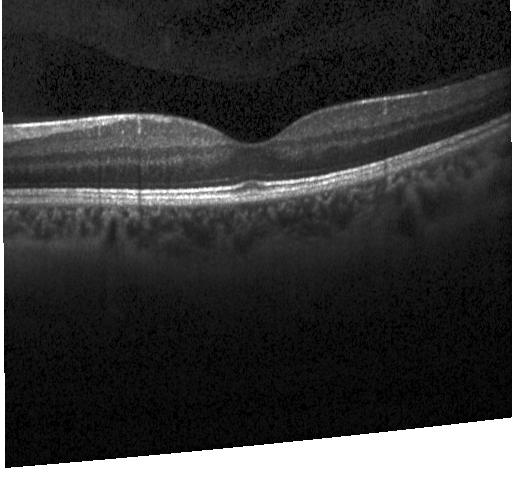

Finding: neither choroidal neovascularization, diabetic macular edema, nor drusen.